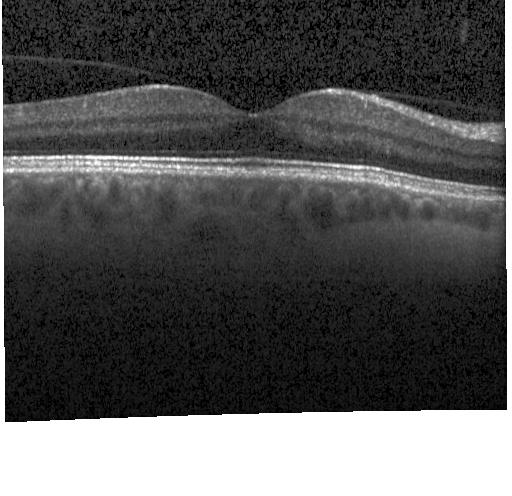

Retinal OCT B-scan · Heidelberg Spectralis · through the macula · spectral-domain OCT.
OCT finding: neither CNV, DME, nor drusen.